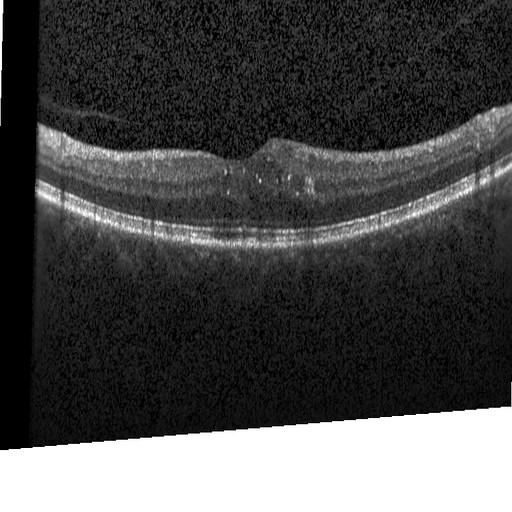 Impression: DME.